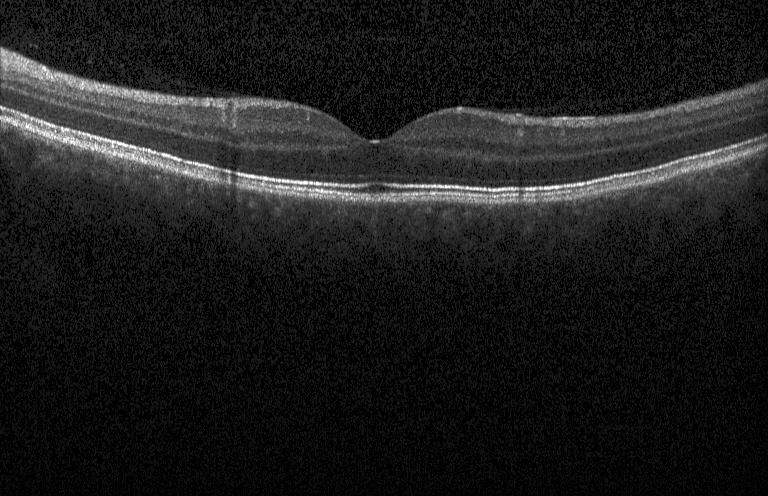
This B-scan demonstrates no CNV, DME, or drusen.